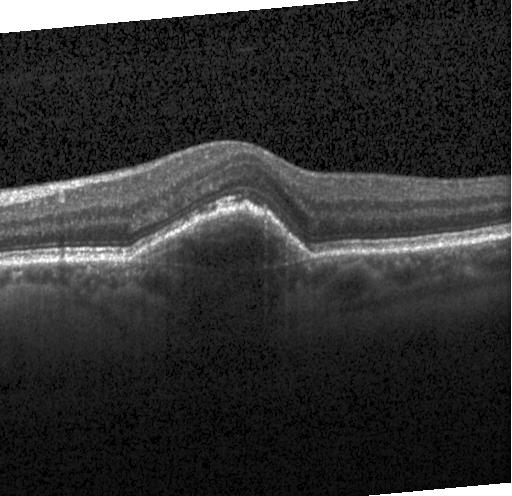 Fovea-centered · retinal OCT B-scan — Diagnosis: choroidal neovascularization (CNV).